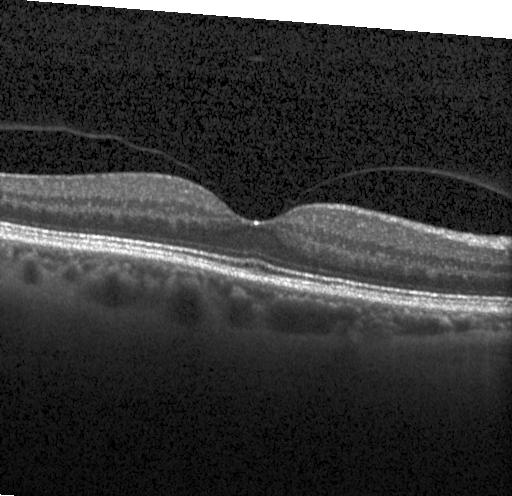

OCT line scan. Finding: no choroidal neovascularization, diabetic macular edema, or drusen.